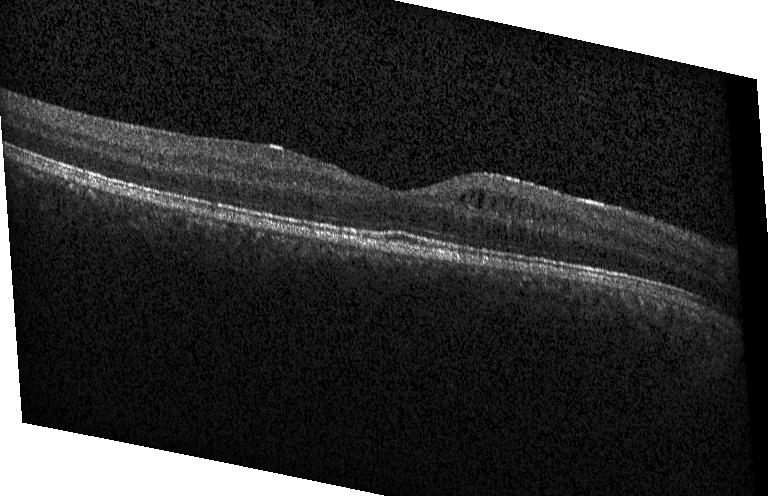
Spectral-domain optical coherence tomography · acquired on a Heidelberg Spectralis · retinal OCT B-scan — OCT finding: DME.